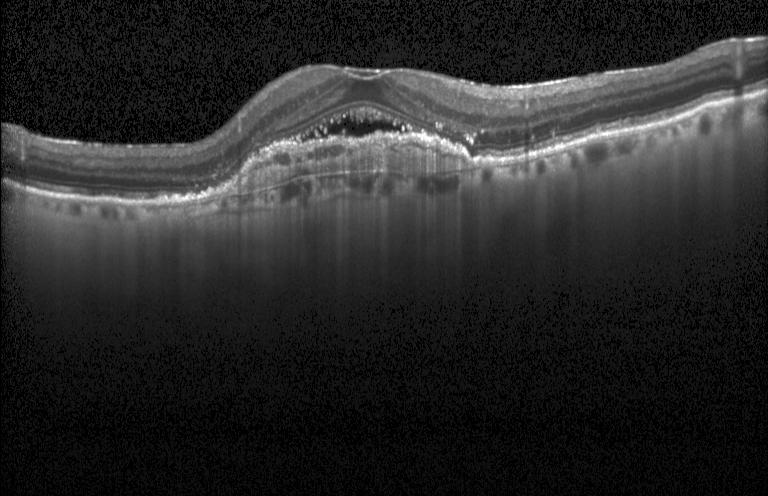 Spectral-domain OCT; Heidelberg Spectralis OCT system; optical coherence tomography scan — OCT finding: choroidal neovascularization.